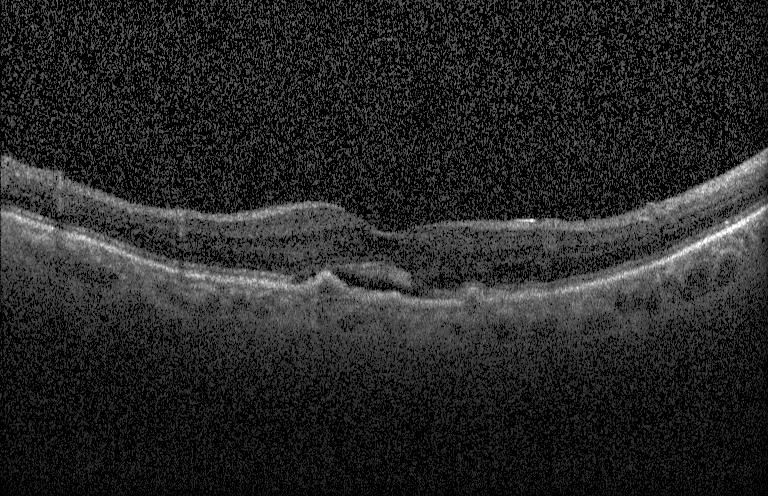
Retinal OCT cross-section — The scan shows CNV.